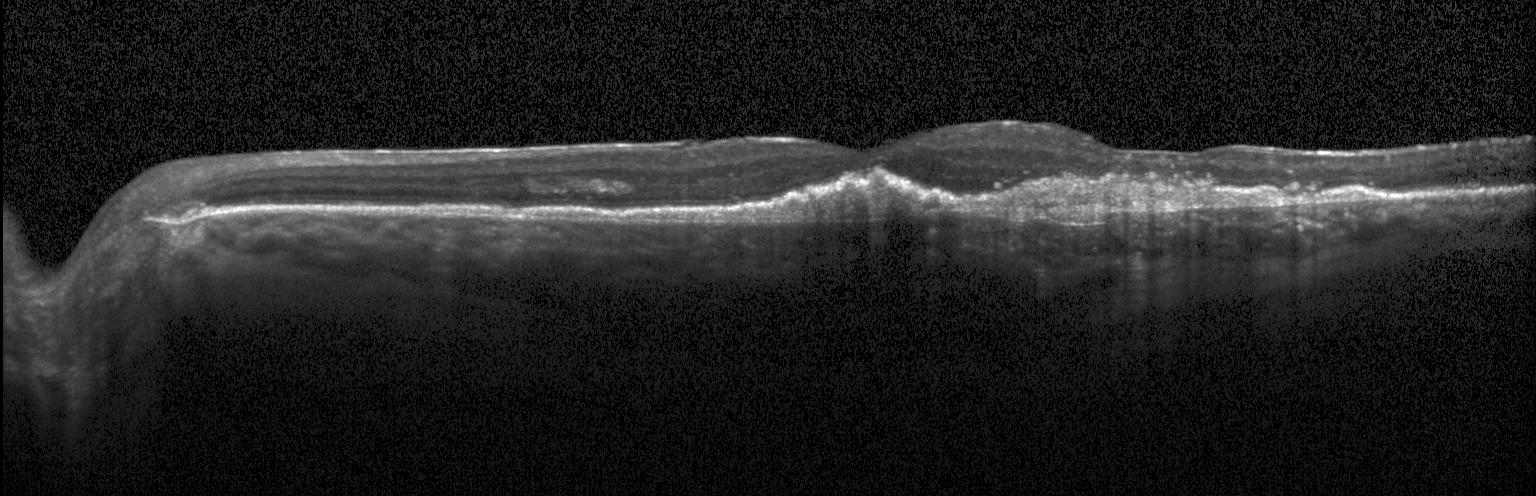

Impression: a choroidal neovascular membrane.